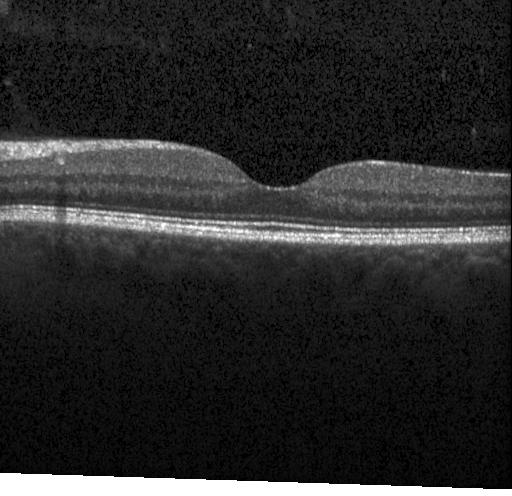
Assessment: neither choroidal neovascularization, diabetic macular edema, nor drusen.